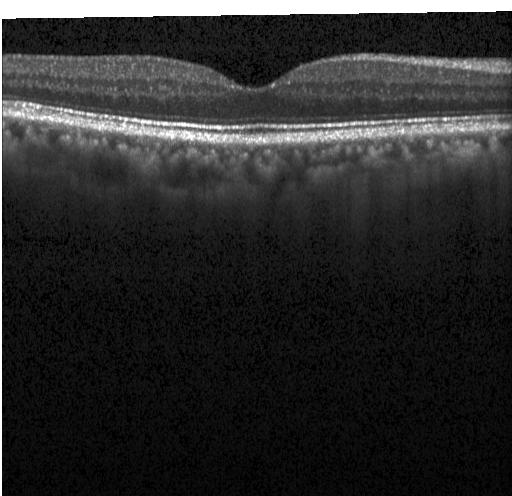 OCT finding: neither CNV, DME, nor drusen.